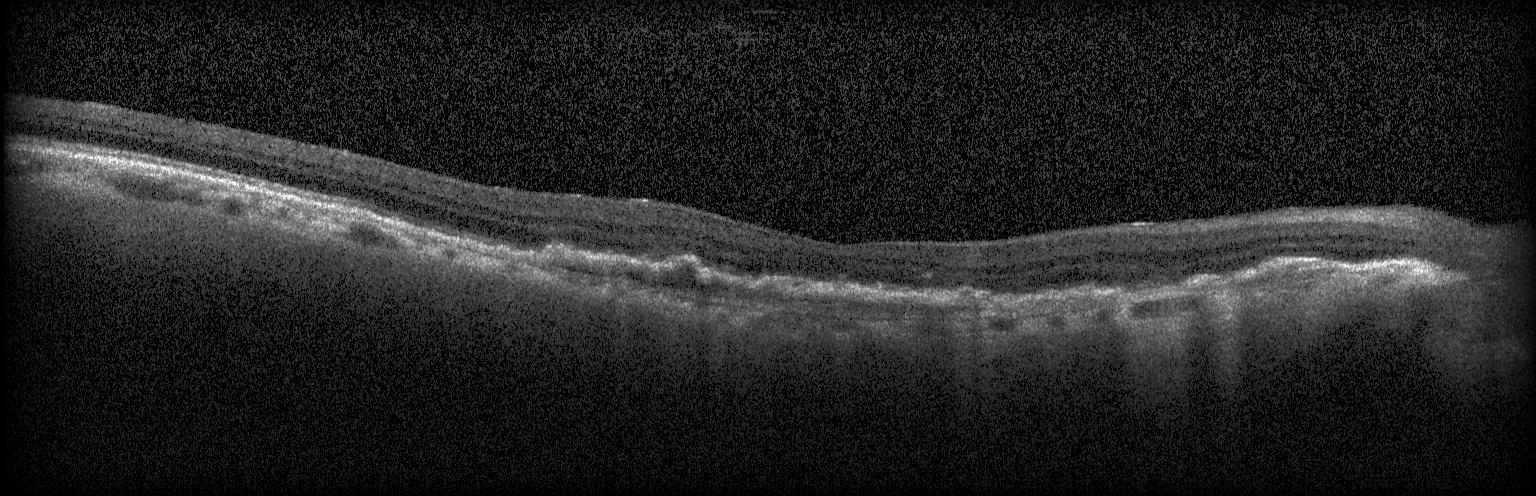 Retinal OCT cross-section; acquired on a Heidelberg Spectralis; spectral-domain optical coherence tomography — A choroidal neovascular membrane.